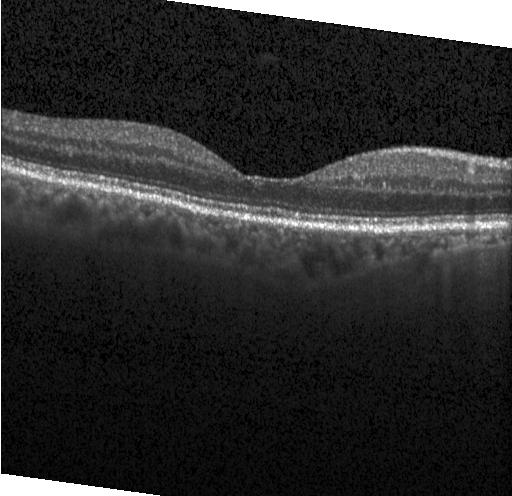 OCT B-scan showing neither choroidal neovascularization, diabetic macular edema, nor drusen.